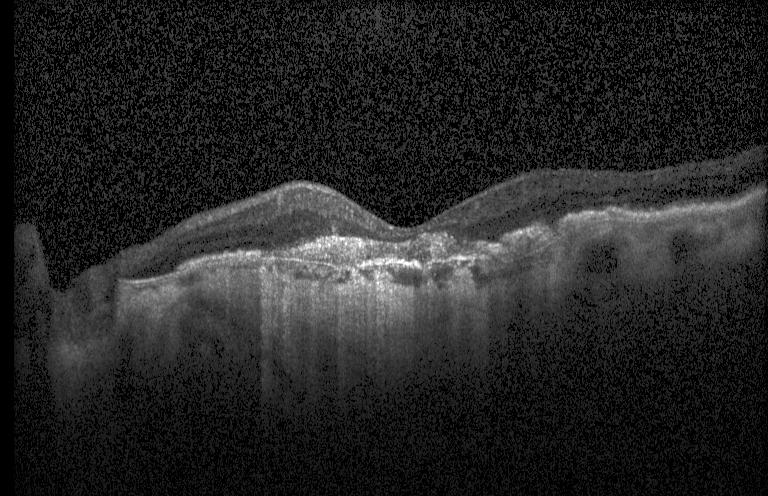 Impression: a choroidal neovascular membrane.